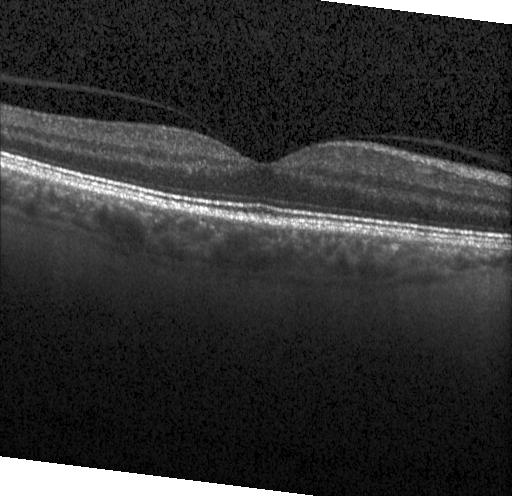 Horizontal scan through the fovea; SD-OCT; optical coherence tomography B-scan; instrument: Heidelberg Spectralis
OCT finding: no CNV, DME, or drusen.